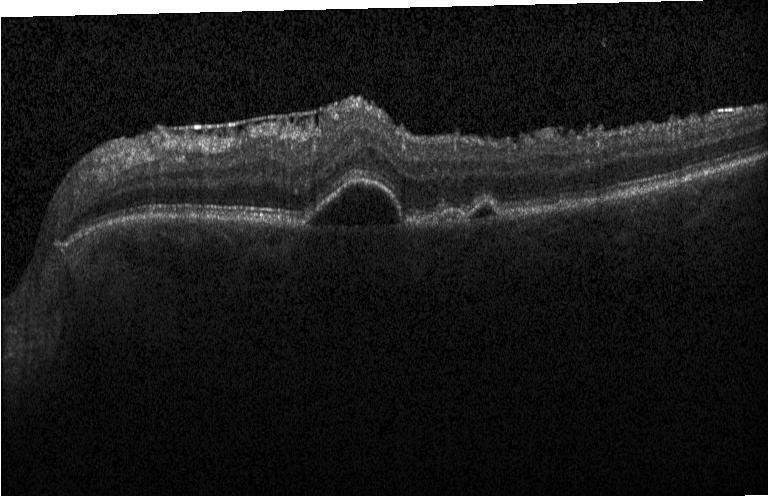 Optical coherence tomography scan; macular scan. Diagnosis: choroidal neovascularization (CNV).